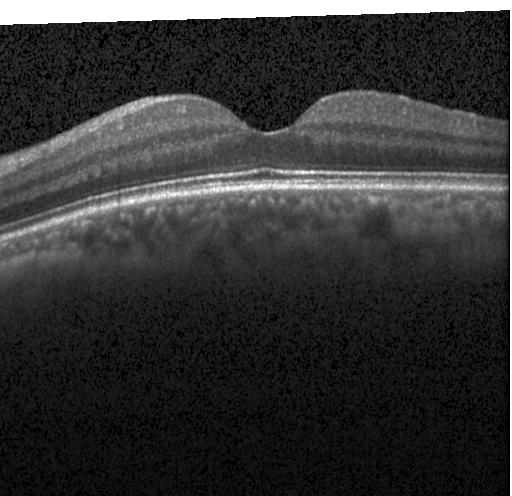 OCT B-scan showing no CNV, no DME, and no drusen.